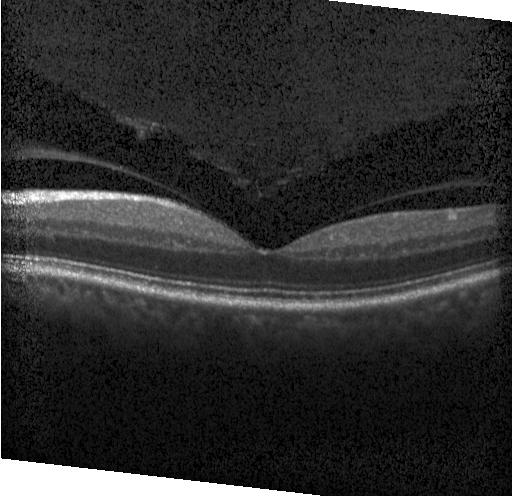
Dx: neither choroidal neovascularization, diabetic macular edema, nor drusen.